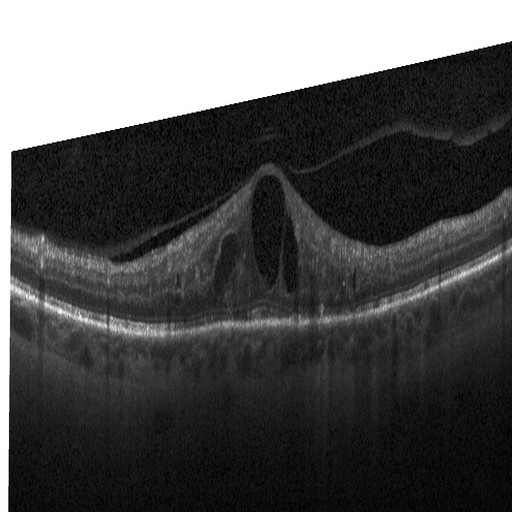 OCT finding: DME.